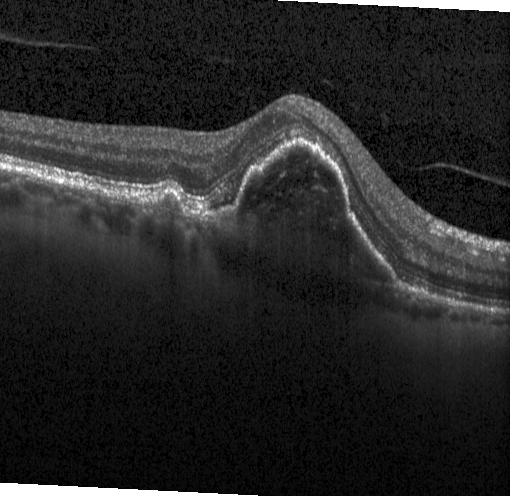

Spectral-domain optical coherence tomography; horizontal scan through the fovea; retinal OCT B-scan; Heidelberg Spectralis
Diagnosis: CNV.